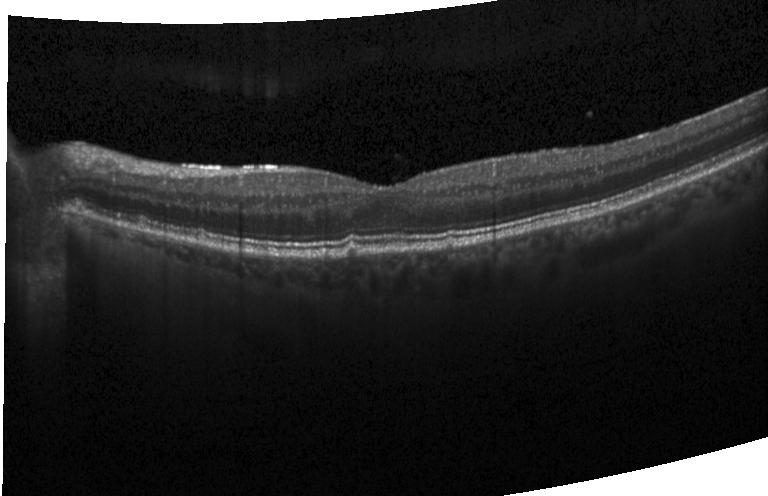

Dx: drusen.